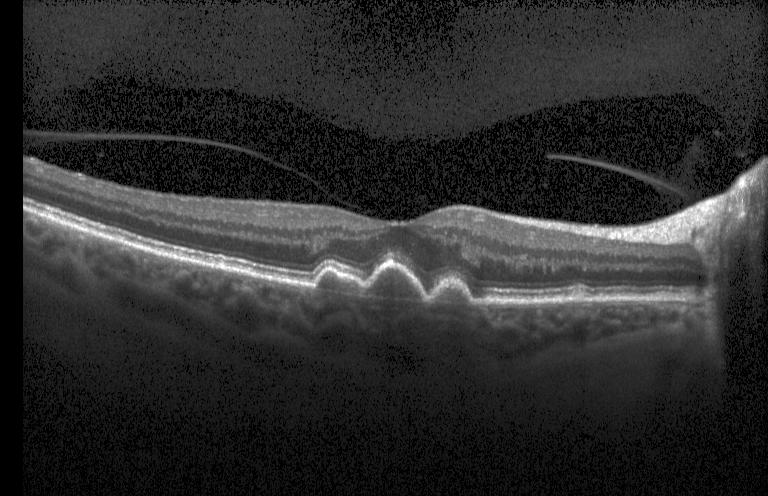
Finding: a choroidal neovascular membrane.